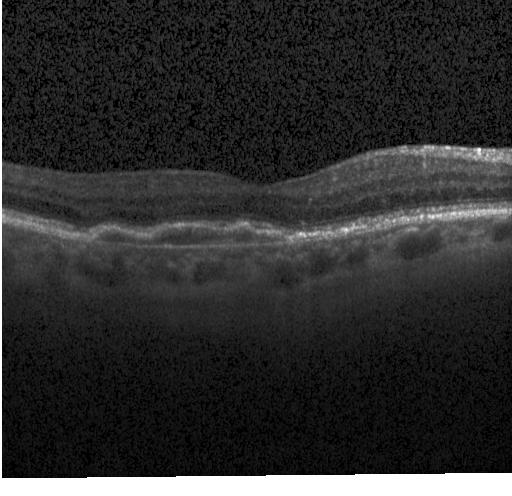 OCT finding: a choroidal neovascular membrane.